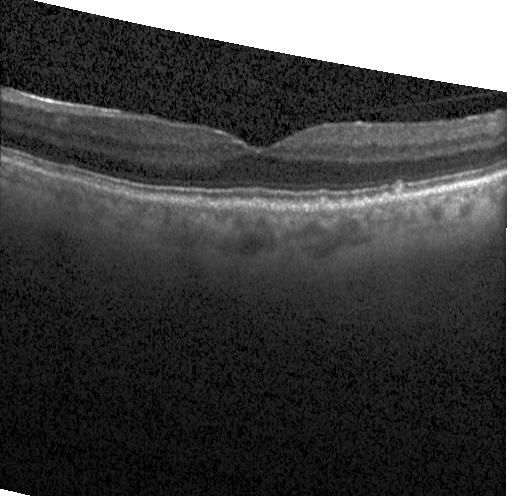
Spectral-domain OCT B-scan: multiple drusen.